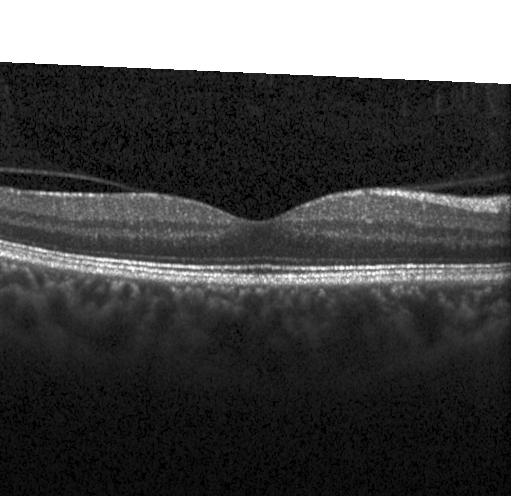 Spectral-domain optical coherence tomography; retinal OCT cross-section.
Finding: no evidence of CNV, DME, or drusen.